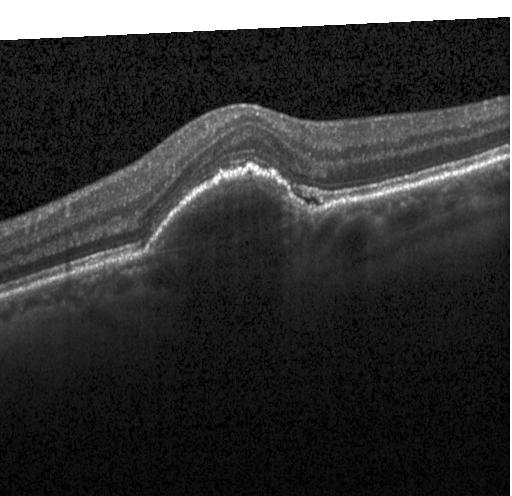

OCT line scan — Assessment: CNV.